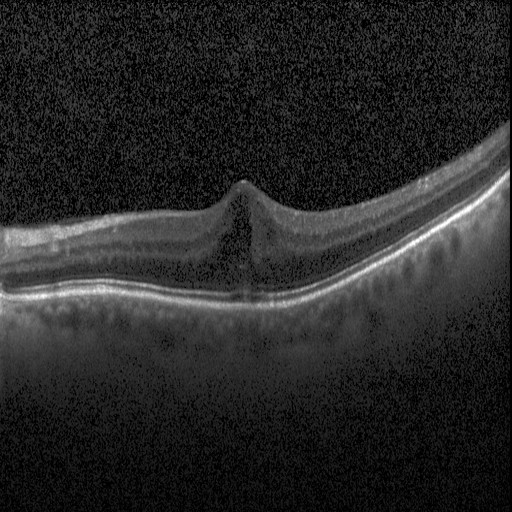 Macular OCT demonstrating diabetic macular edema.